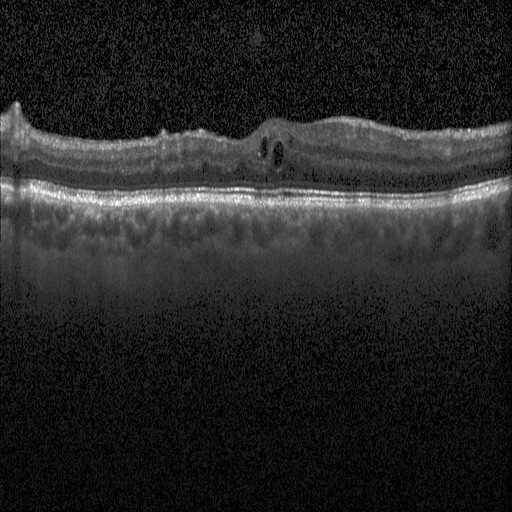
Heidelberg Spectralis. OCT B-scan. Centered on the fovea — Diagnosis: DME.